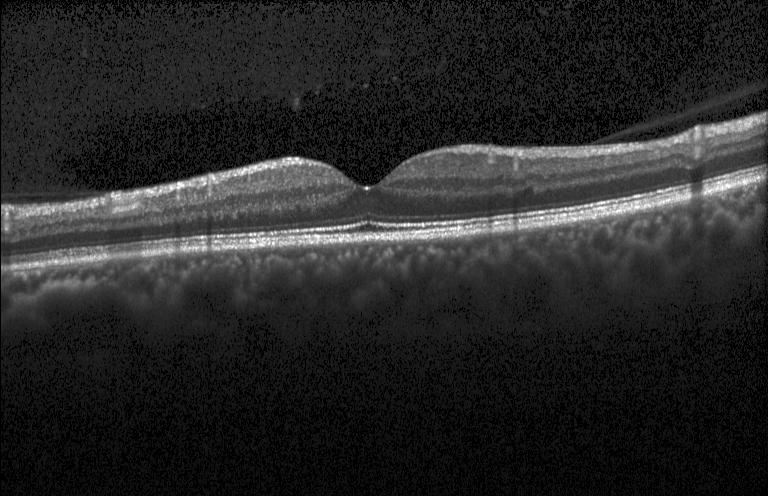

Finding: neither choroidal neovascularization, diabetic macular edema, nor drusen.